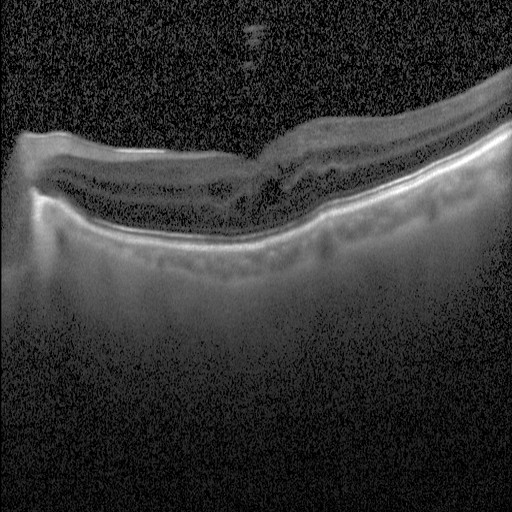

Instrument: Heidelberg Spectralis · SD-OCT · macular scan · retinal OCT B-scan. Diagnosis: diabetic macular edema.